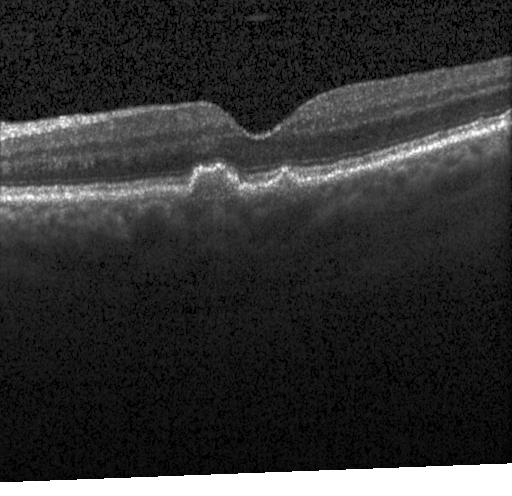
Heidelberg Spectralis OCT system · spectral-domain optical coherence tomography · OCT B-scan. Impression: sub-RPE drusenoid deposits.